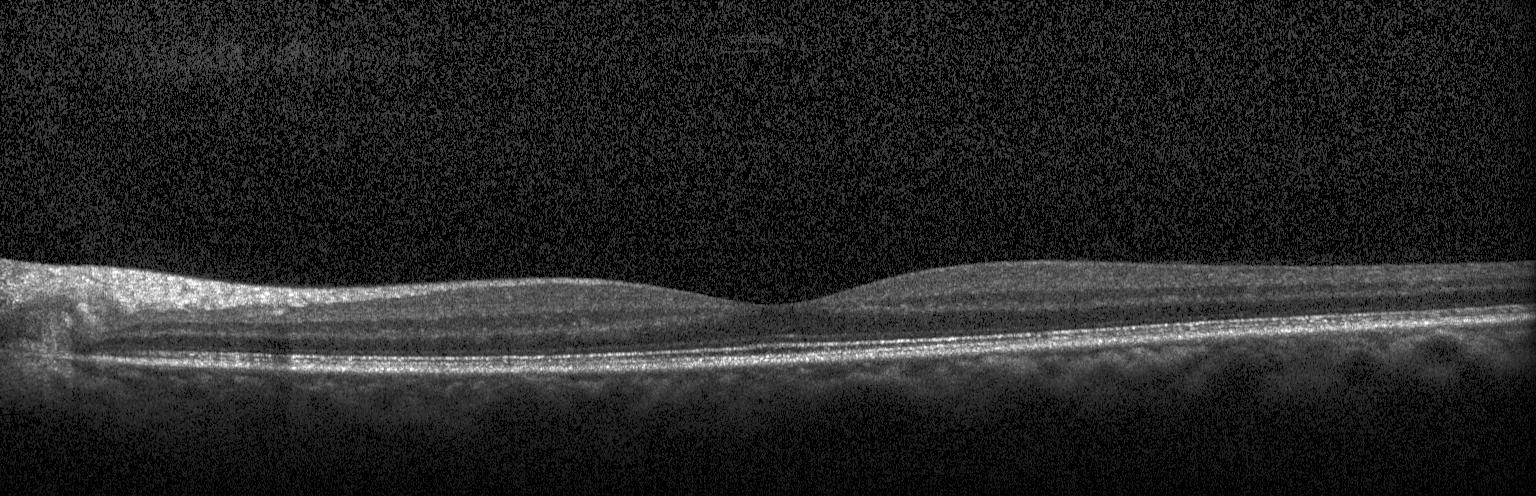

Spectral-domain OCT B-scan: neither CNV, DME, nor drusen.